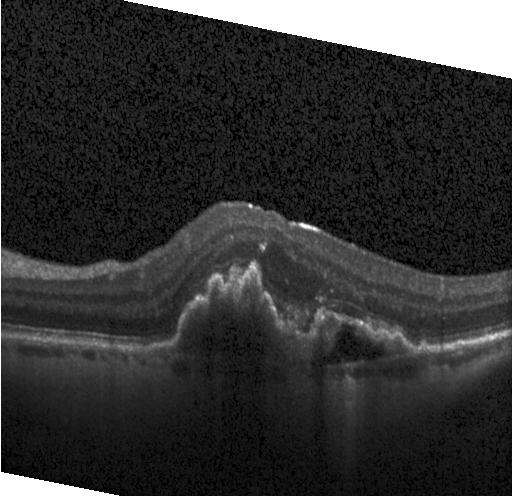 SD-OCT · optical coherence tomography B-scan
This B-scan demonstrates a choroidal neovascular membrane.